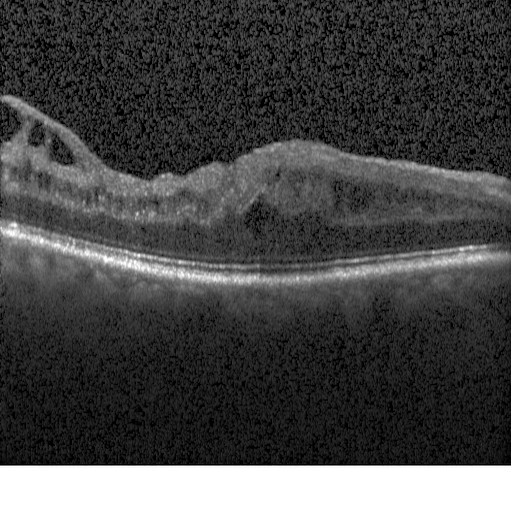
Through the macula · SD-OCT · optical coherence tomography scan · Heidelberg Spectralis OCT system. Diabetic macular edema.